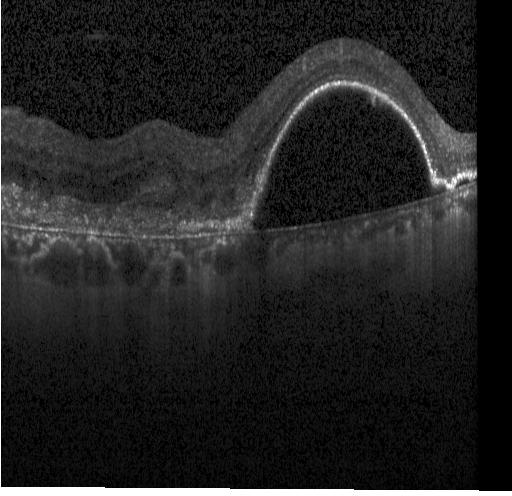
Through the macula · acquired on a Heidelberg Spectralis · spectral-domain OCT · OCT B-scan — Assessment: a choroidal neovascular membrane.